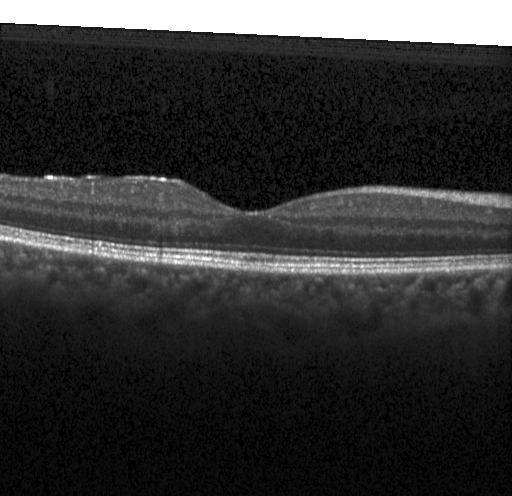
Assessment: no evidence of choroidal neovascularization, diabetic macular edema, or drusen.